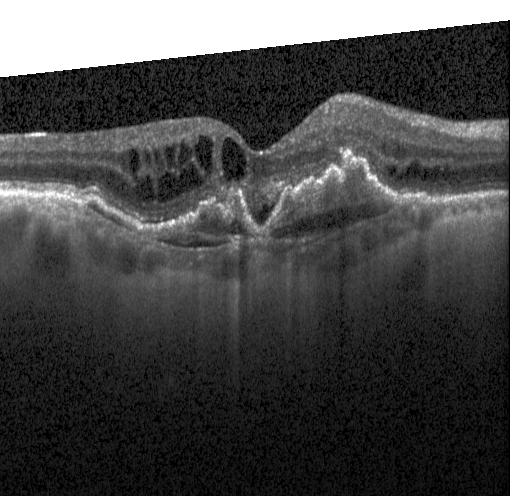

Spectral-domain OCT, retinal OCT cross-section.
The scan shows a choroidal neovascular membrane.